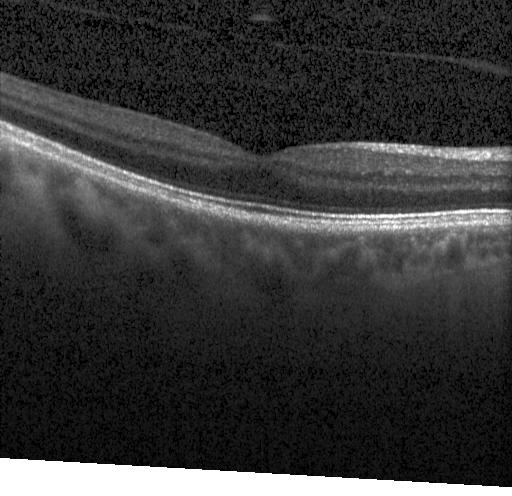

Heidelberg Spectralis OCT system, optical coherence tomography scan.
Finding: neither choroidal neovascularization, diabetic macular edema, nor drusen.